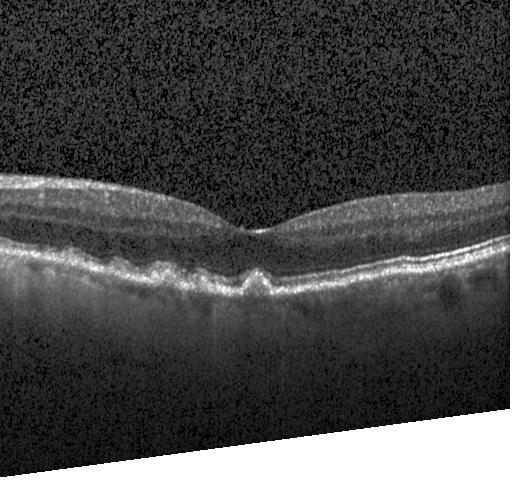

SD-OCT. Retinal OCT B-scan. Fovea-centered. Acquired on a Heidelberg Spectralis — Impression: sub-RPE drusenoid deposits.